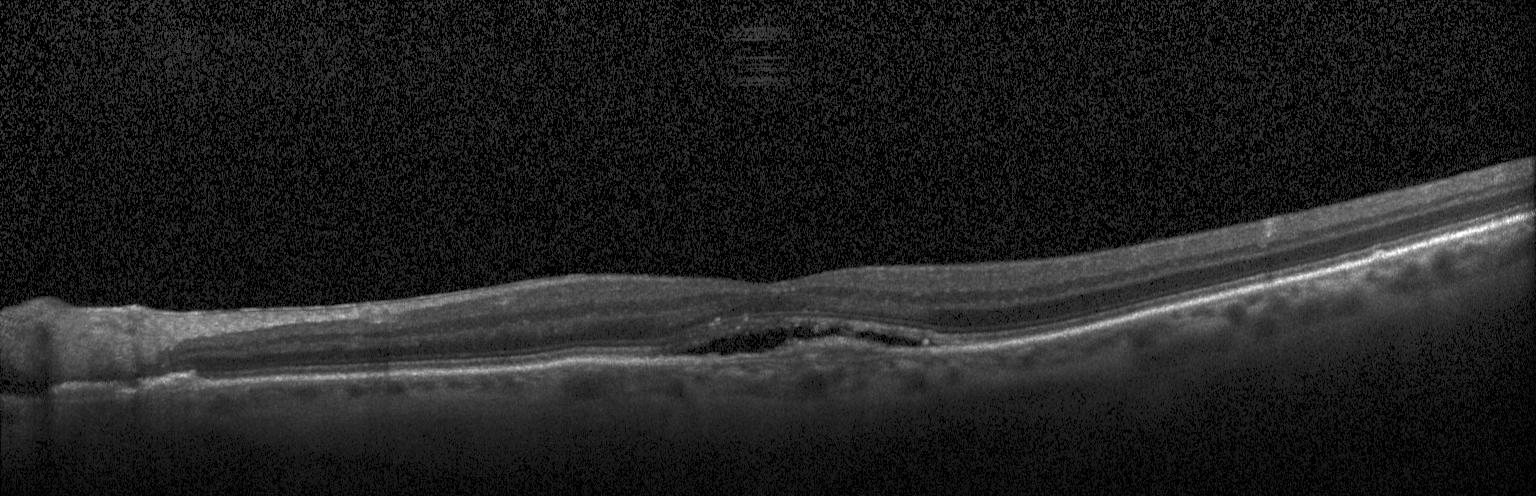 Spectral-domain OCT; retinal OCT cross-section. Assessment: a choroidal neovascular membrane.